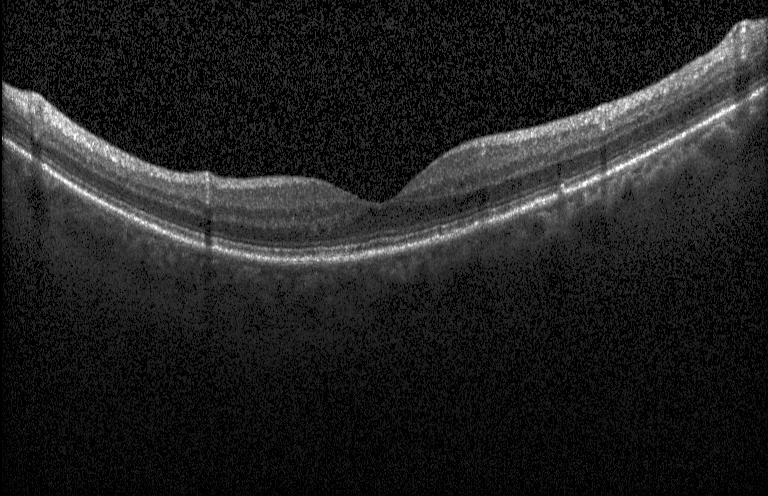
Optical coherence tomography B-scan.
The scan shows no choroidal neovascularization, diabetic macular edema, or drusen.